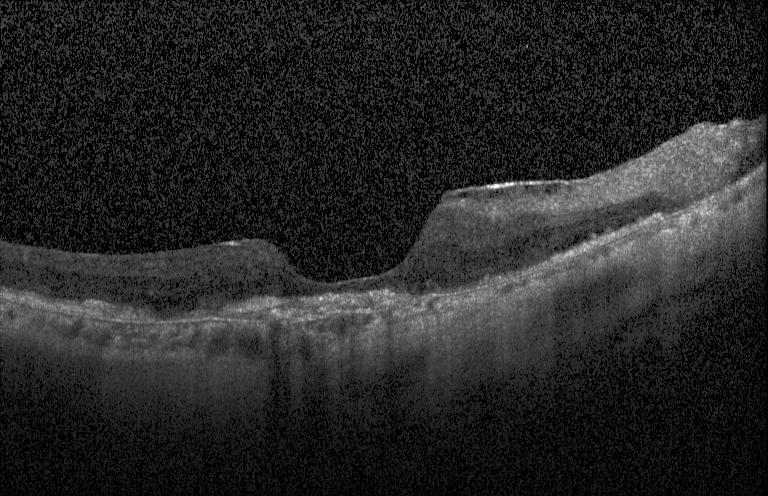 Instrument: Heidelberg Spectralis · horizontal scan through the fovea · optical coherence tomography B-scan.
Finding: choroidal neovascularization (CNV).